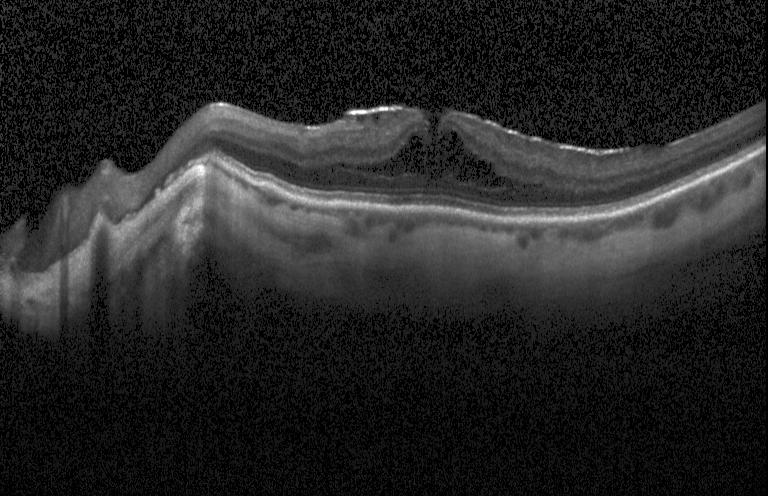
Finding: diabetic macular edema.